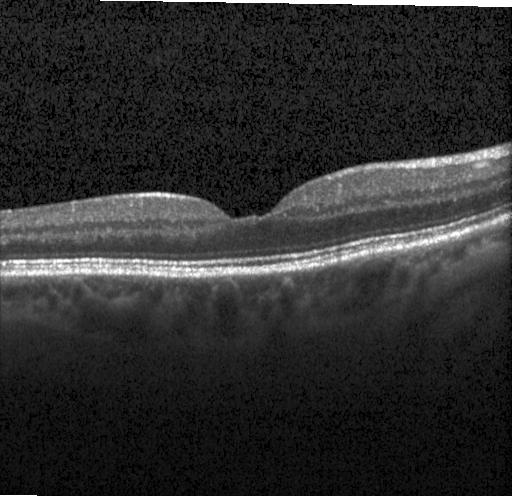
Retinal OCT cross-section — OCT finding: no choroidal neovascularization, diabetic macular edema, or drusen.